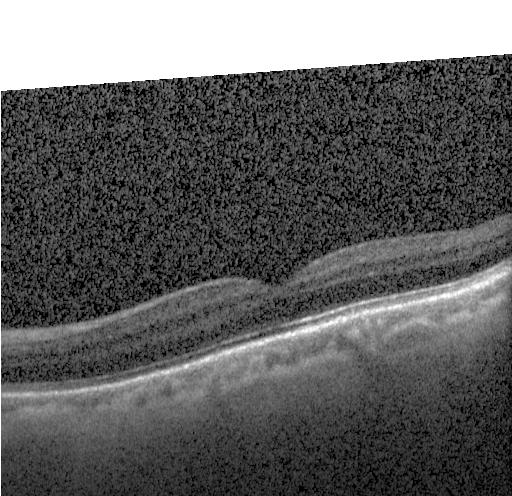 Optical coherence tomography B-scan.
Impression: no evidence of CNV, DME, or drusen.